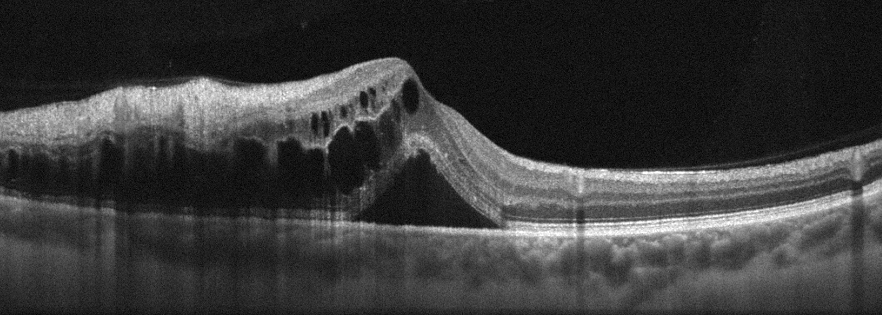
Finding: RVO.